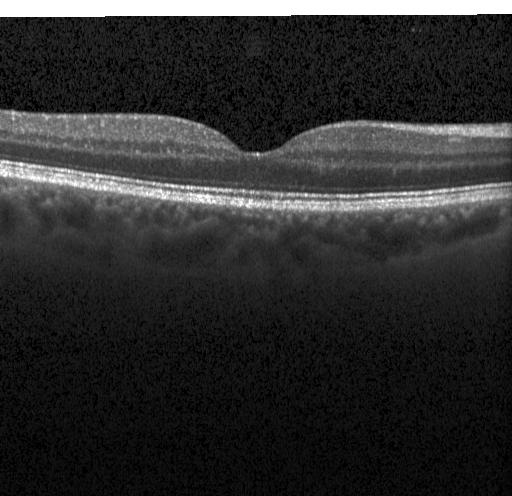 Finding: neither choroidal neovascularization, diabetic macular edema, nor drusen.